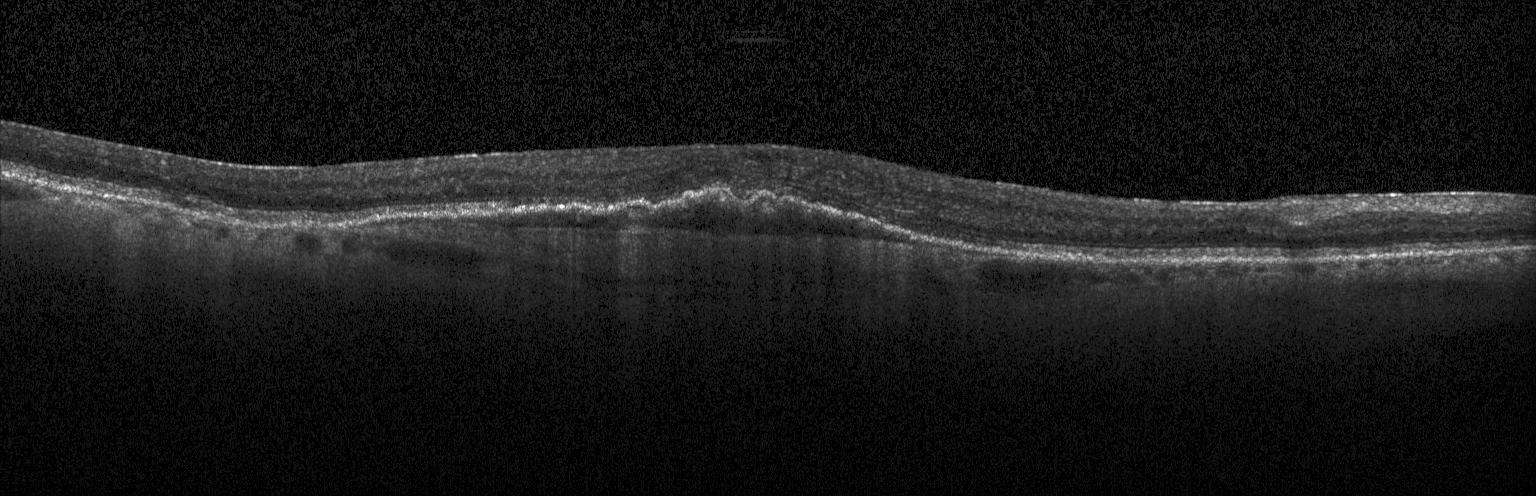 Retinal OCT B-scan
Impression: a choroidal neovascular membrane.